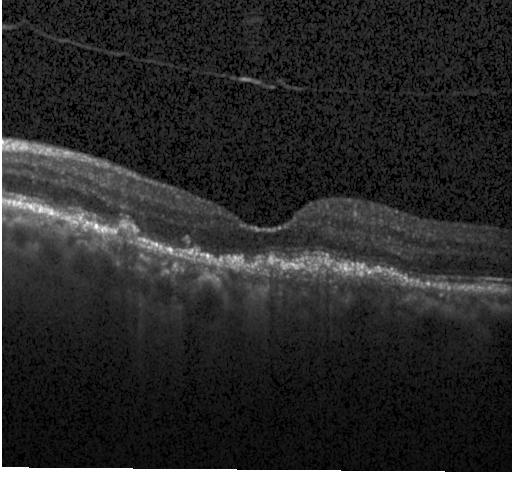

OCT finding: CNV.